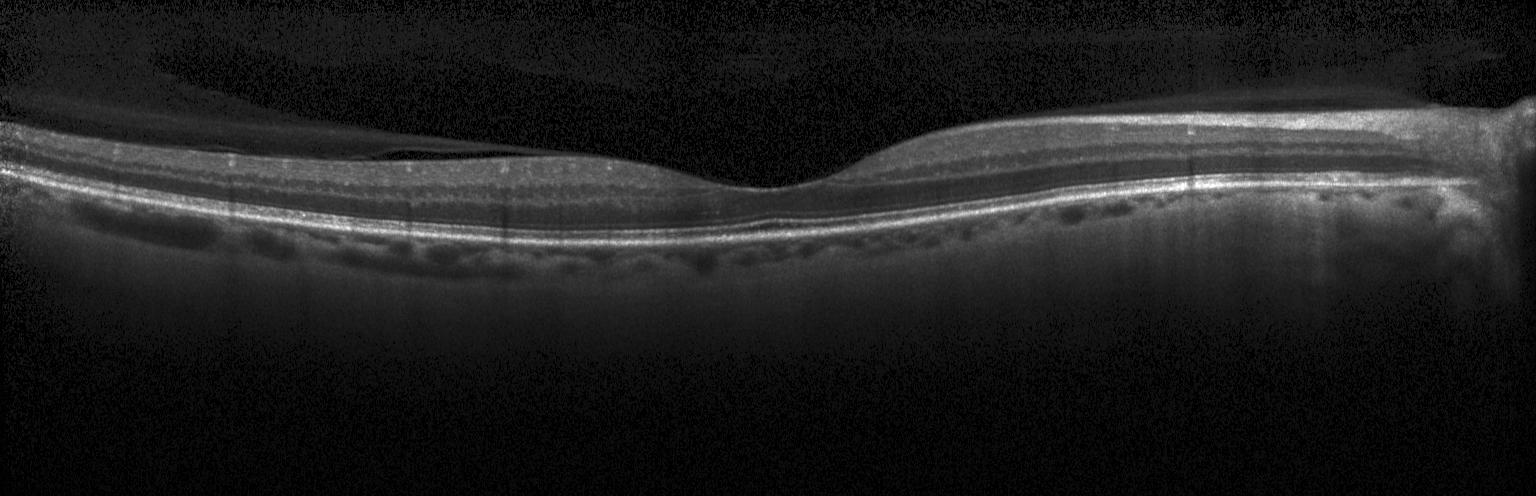 Centered on the fovea; optical coherence tomography scan. Assessment: neither choroidal neovascularization, diabetic macular edema, nor drusen.